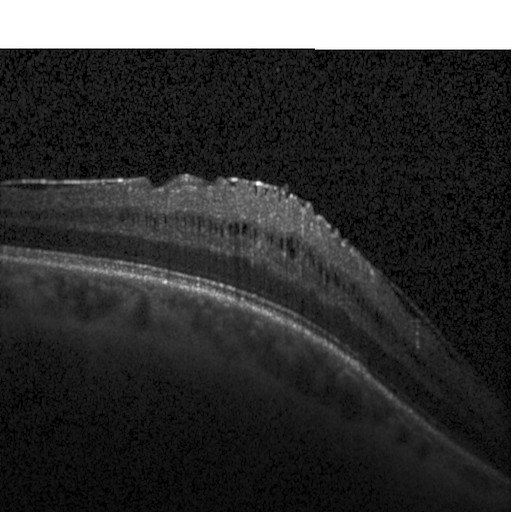

Diagnosis: DME.